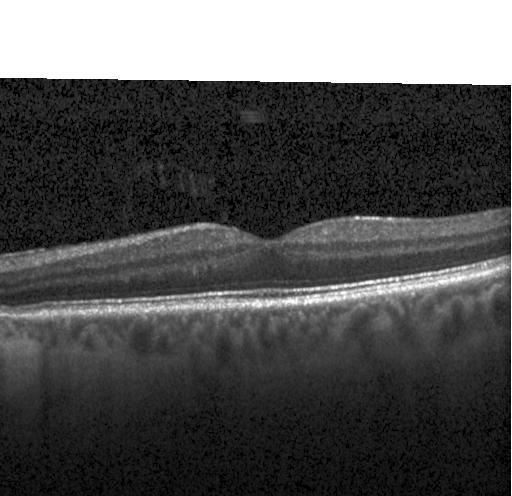
OCT scan showing no choroidal neovascularization, diabetic macular edema, or drusen.